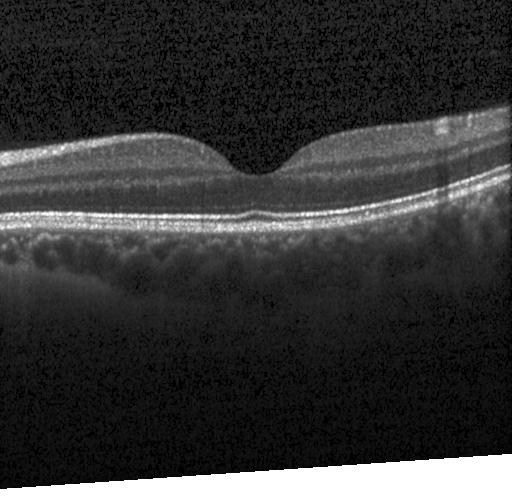

Optical coherence tomography B-scan. Impression: no choroidal neovascularization, diabetic macular edema, or drusen.